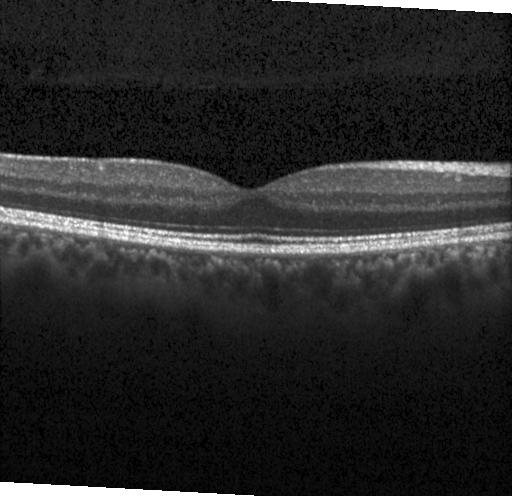
Optical coherence tomography scan.
Dx: no evidence of choroidal neovascularization, diabetic macular edema, or drusen.